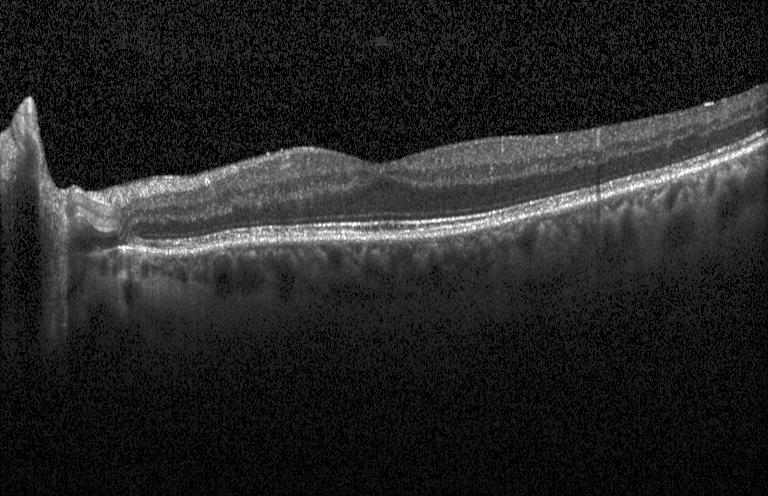
Finding: no evidence of choroidal neovascularization, diabetic macular edema, or drusen.